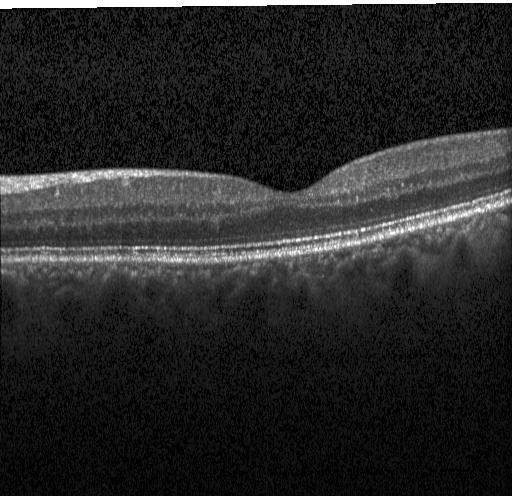

Acquired on a Heidelberg Spectralis, through the macula, retinal OCT cross-section, spectral-domain OCT
Finding: no evidence of choroidal neovascularization, diabetic macular edema, or drusen.